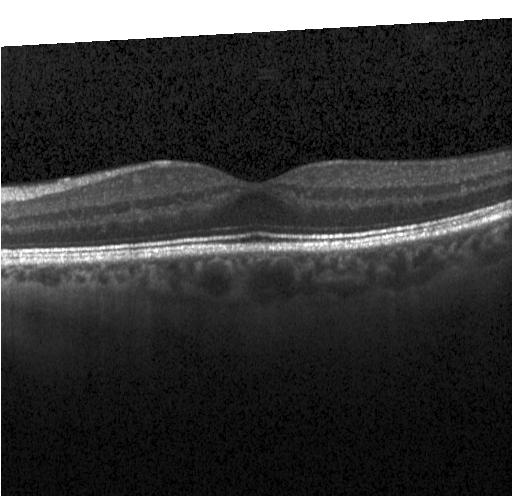

Through the macula, OCT line scan.
Diagnosis: no choroidal neovascularization, no diabetic macular edema, and no drusen.